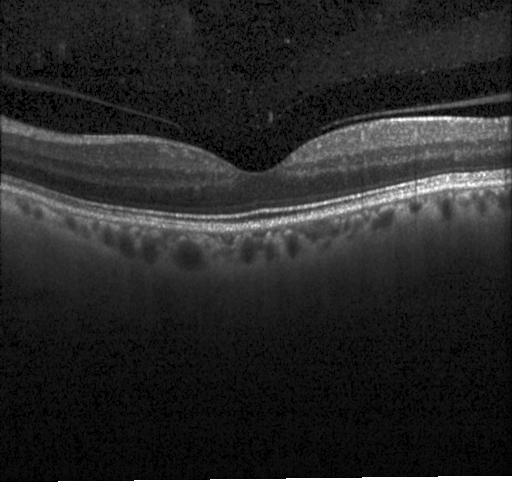
OCT finding: no evidence of choroidal neovascularization, diabetic macular edema, or drusen.